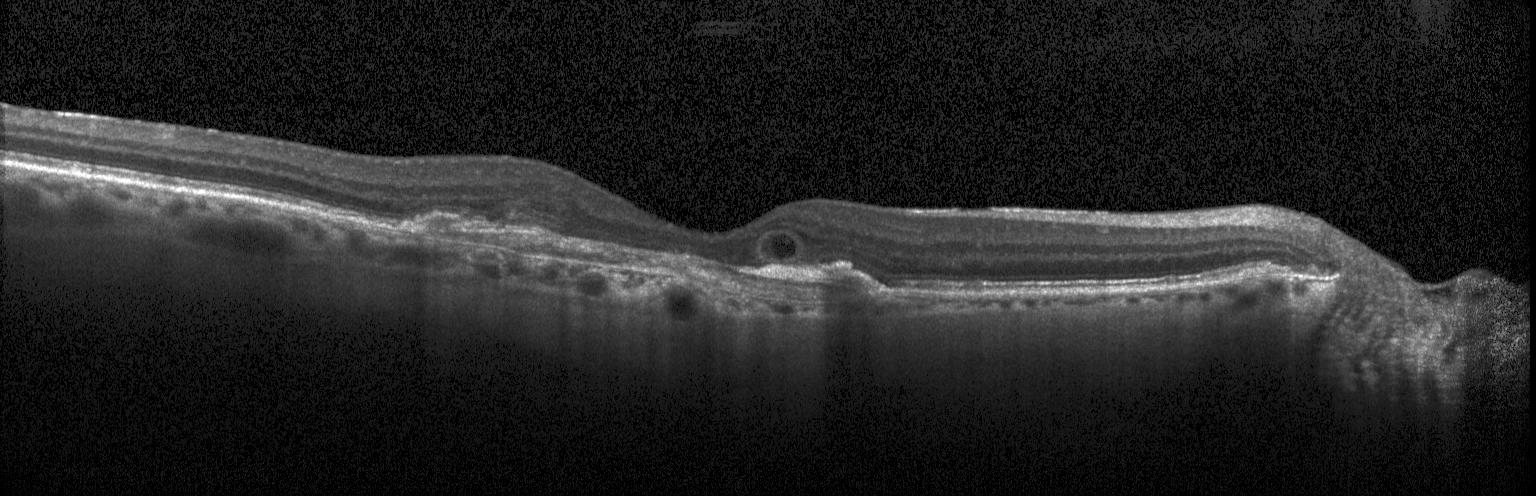 Spectral-domain optical coherence tomography. OCT B-scan. Through the macula. Choroidal neovascularization (CNV).